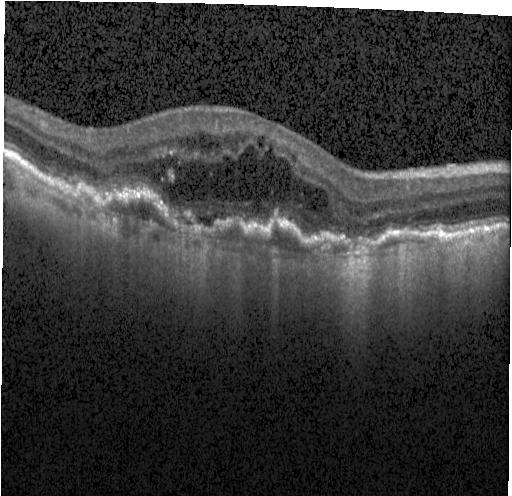 Finding: a choroidal neovascular membrane.